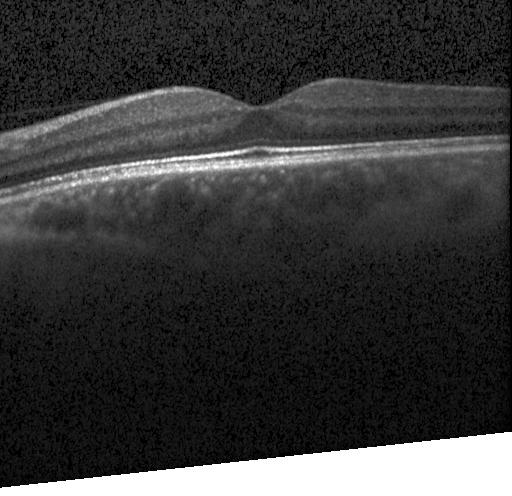
Through the macula, Heidelberg Spectralis, optical coherence tomography scan, spectral-domain OCT. Diagnosis: no choroidal neovascularization, diabetic macular edema, or drusen.